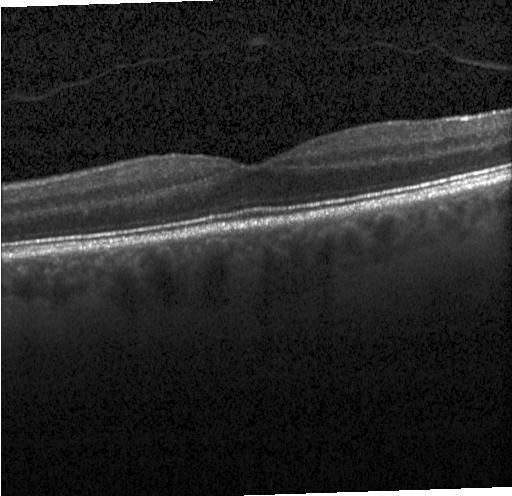

Retinal OCT B-scan. Dx: no evidence of CNV, DME, or drusen.